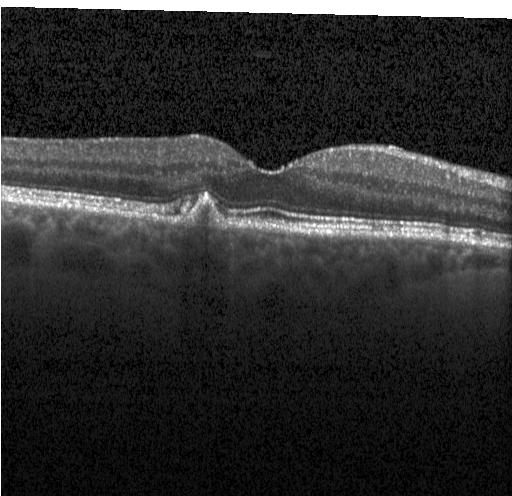

Optical coherence tomography scan. Instrument: Heidelberg Spectralis — Macular OCT: a choroidal neovascular membrane.